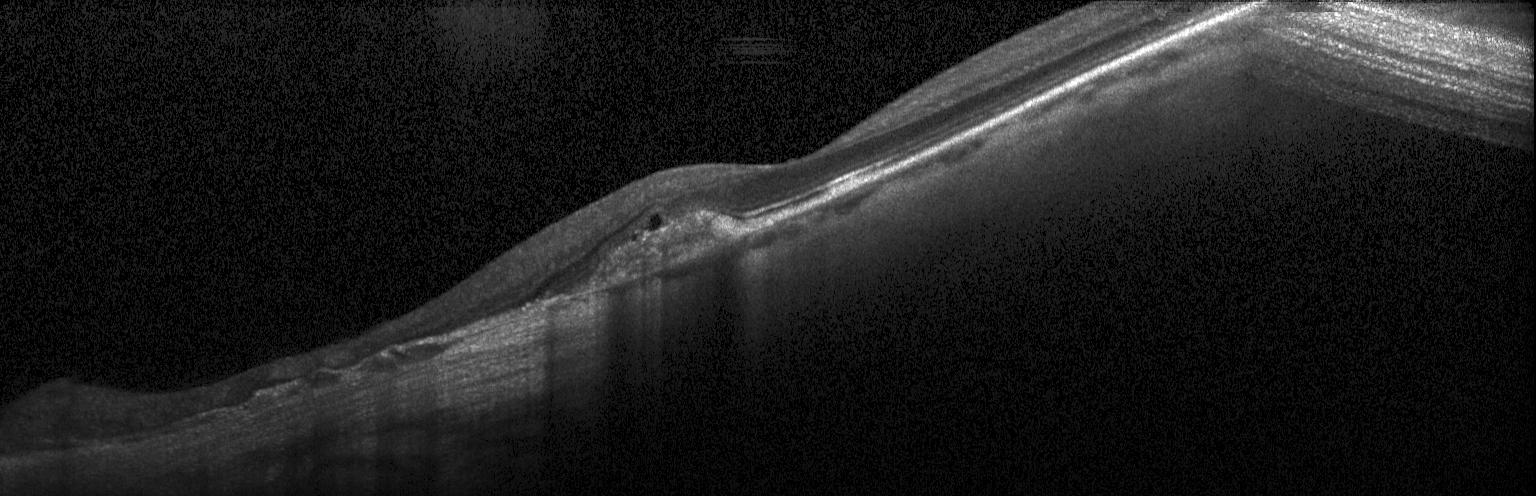 Spectral-domain optical coherence tomography; fovea-centered; OCT B-scan; Heidelberg Spectralis. Finding: choroidal neovascularization (CNV).